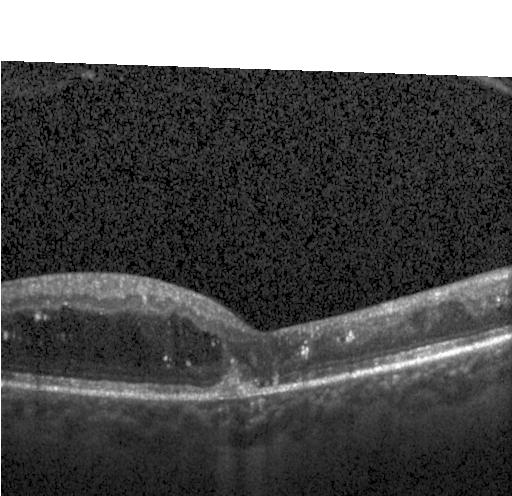
Spectral-domain optical coherence tomography; Heidelberg Spectralis; retinal OCT cross-section; fovea-centered. Macular OCT: DME.